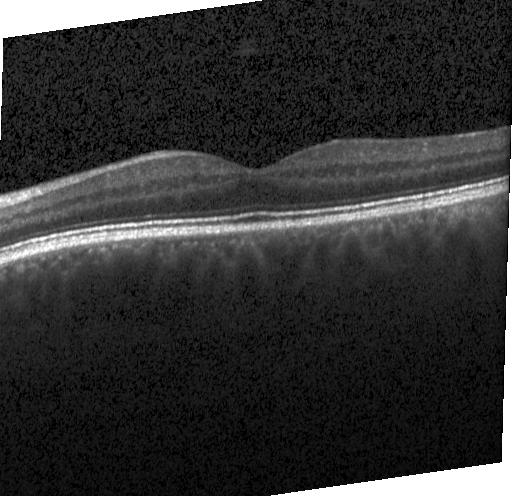
SD-OCT · centered on the fovea · OCT B-scan.
Impression: no CNV, no DME, and no drusen.